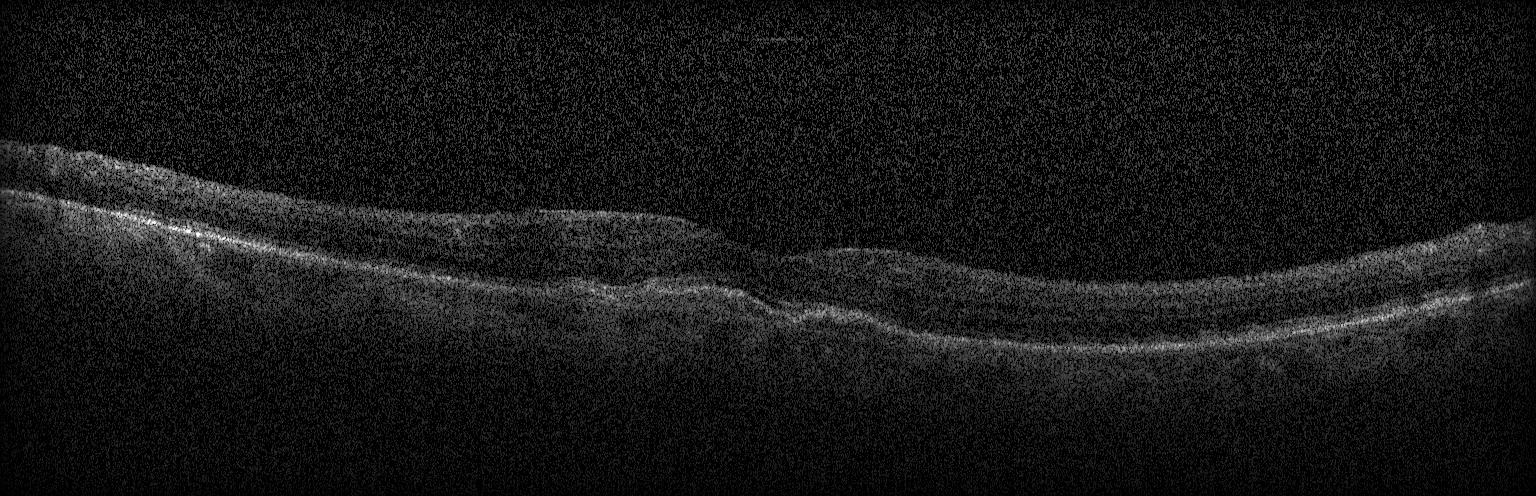

OCT finding: a choroidal neovascular membrane.